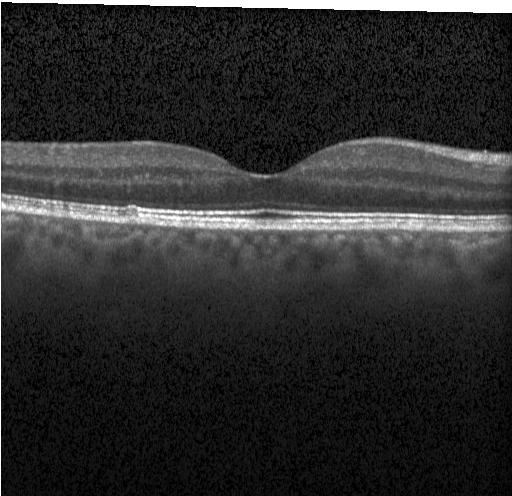 Acquired on a Heidelberg Spectralis. Retinal OCT B-scan. Horizontal scan through the fovea. Spectral-domain OCT.
The scan shows drusen.